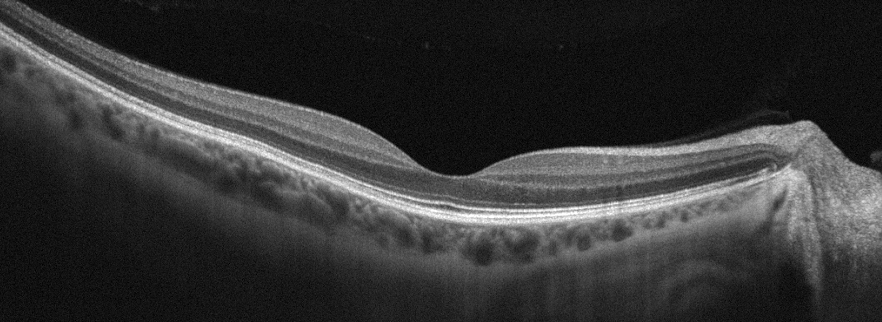 Retinal OCT B-scan; oculus dexter; acquired on an Optovue Avanti RTVue XR; macular scan. Diagnosis: no evidence of AMD, DME, ERM, RAO, RVO, or VID.